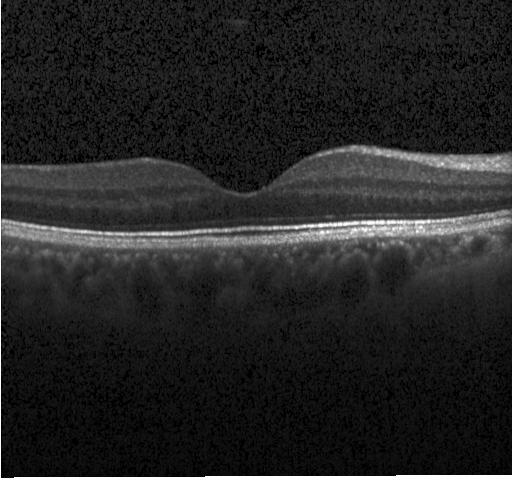
The scan shows no evidence of CNV, DME, or drusen.